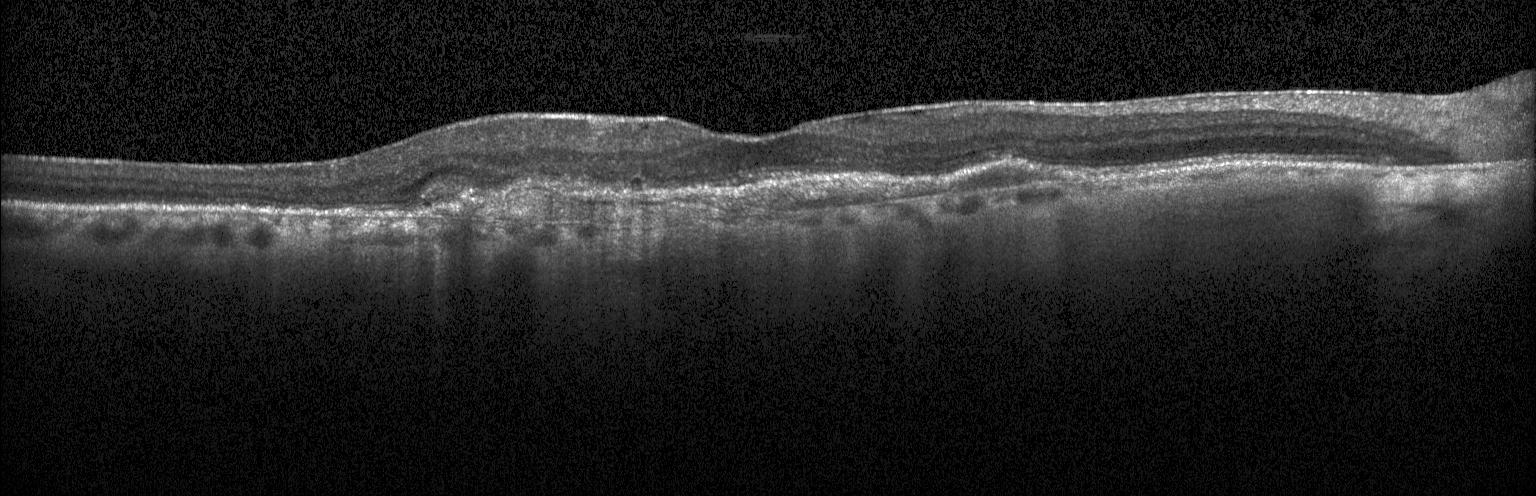

Impression: a choroidal neovascular membrane.